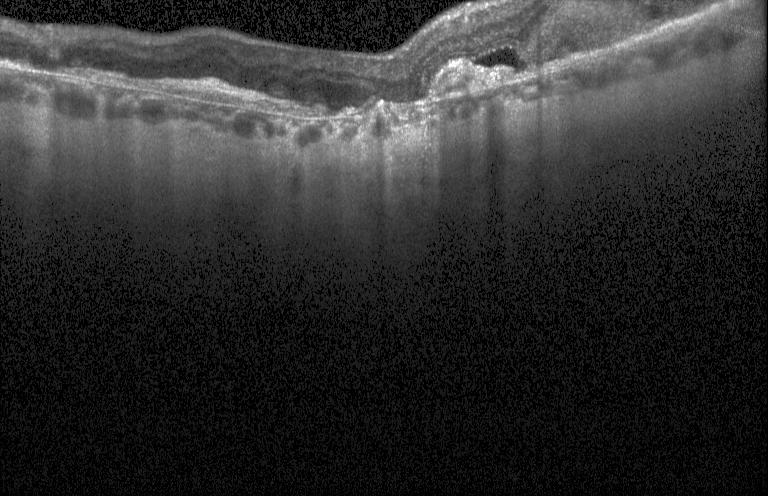 Centered on the fovea, OCT B-scan.
Diagnosis: CNV.